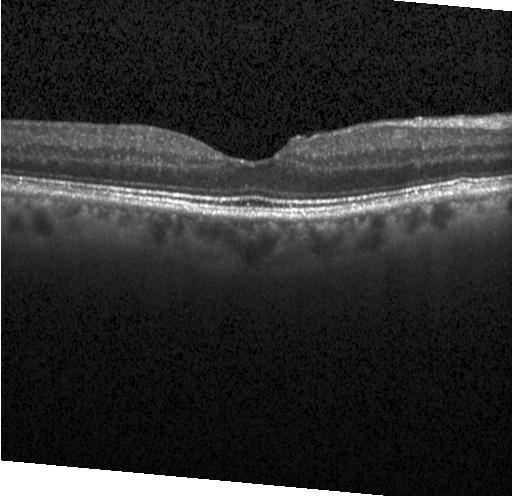
Macular OCT demonstrating neither CNV, DME, nor drusen.